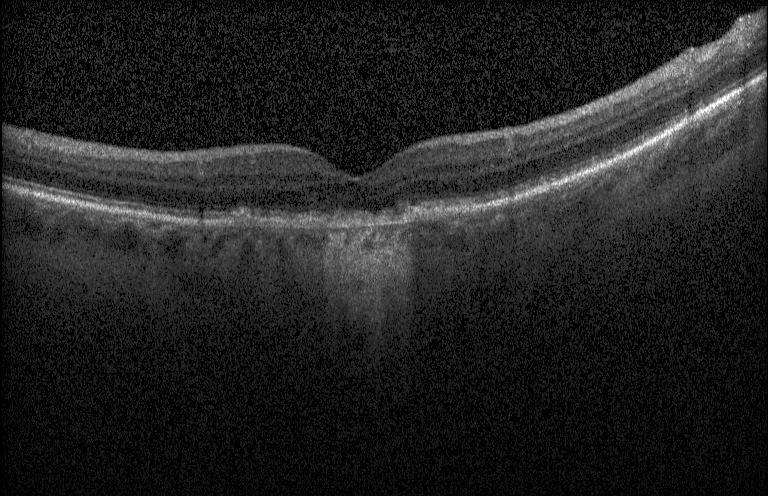

The scan shows a choroidal neovascular membrane.